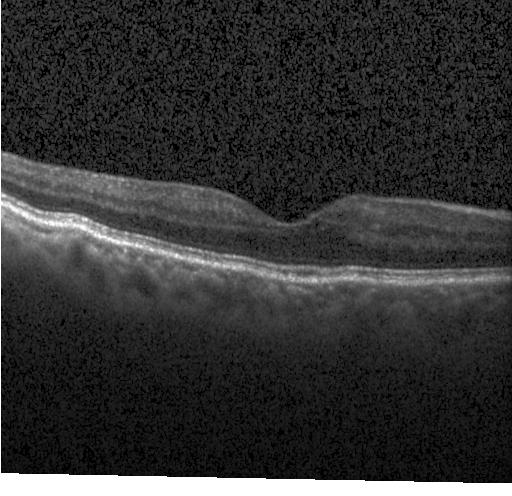
Optical coherence tomography scan, spectral-domain optical coherence tomography, centered on the fovea, Heidelberg Spectralis OCT system.
Dx: neither choroidal neovascularization, diabetic macular edema, nor drusen.